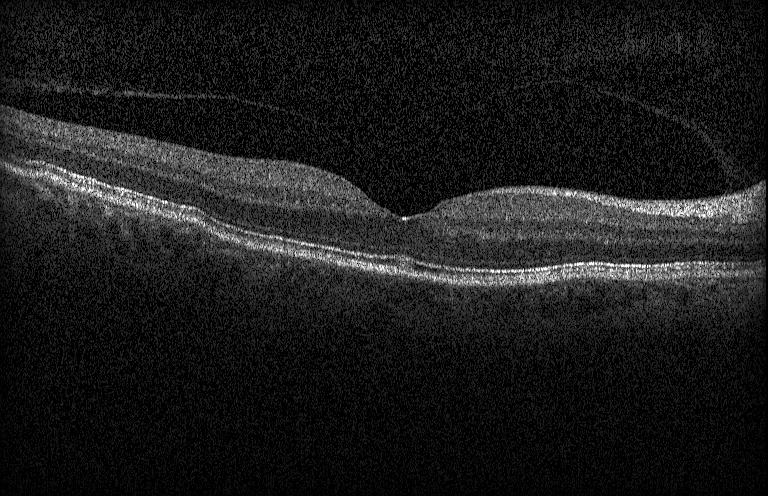

No choroidal neovascularization, diabetic macular edema, or drusen.